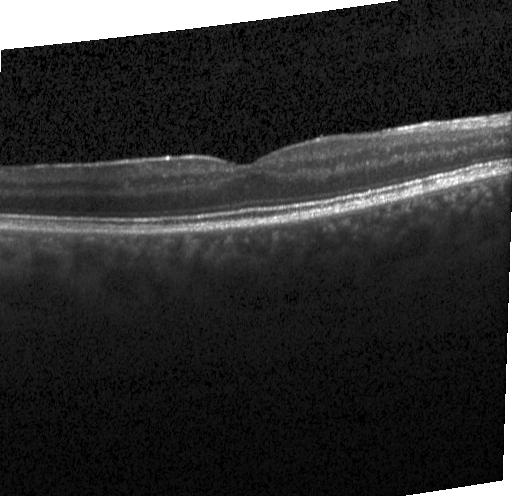

OCT B-scan showing no evidence of choroidal neovascularization, diabetic macular edema, or drusen.